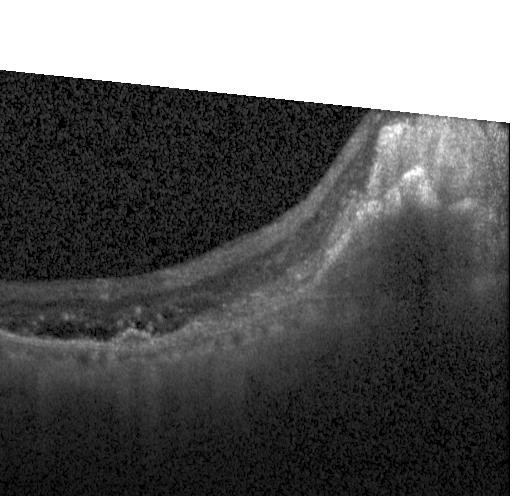
Macular OCT demonstrating a choroidal neovascular membrane.